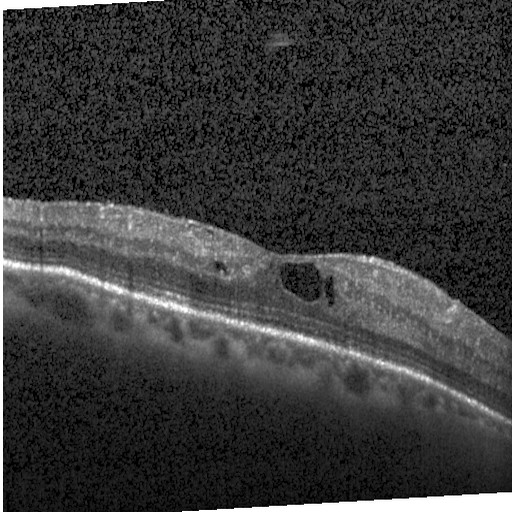

OCT B-scan · centered on the fovea
Diagnosis: DME.